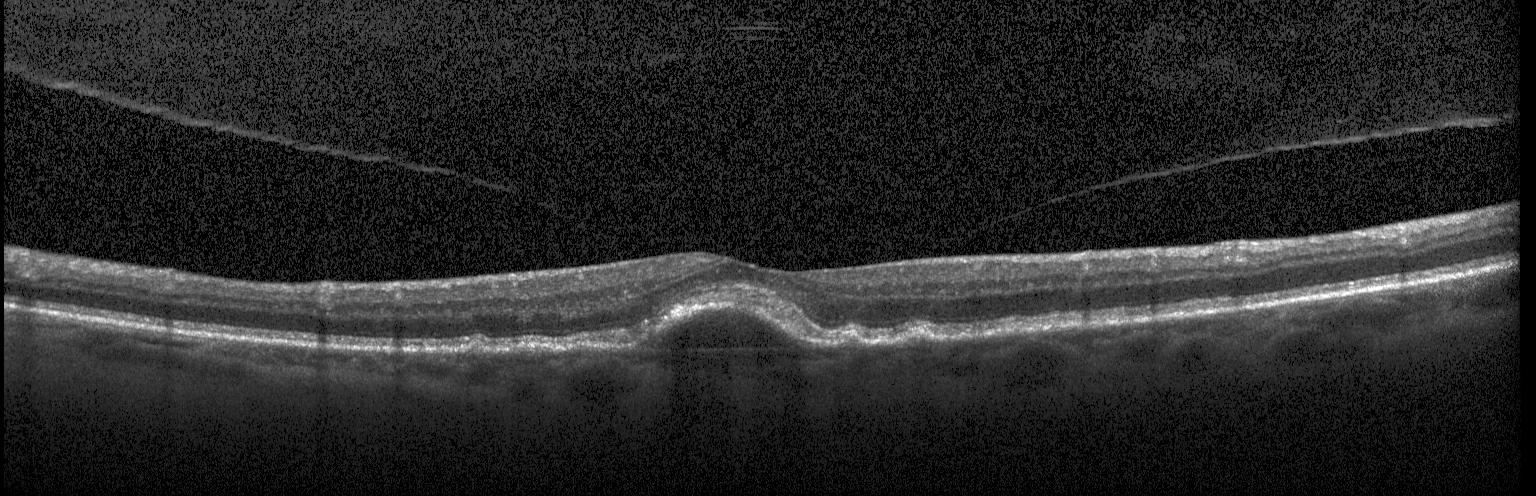 Retinal OCT cross-section · spectral-domain optical coherence tomography · fovea-centered — Diagnosis: CNV.